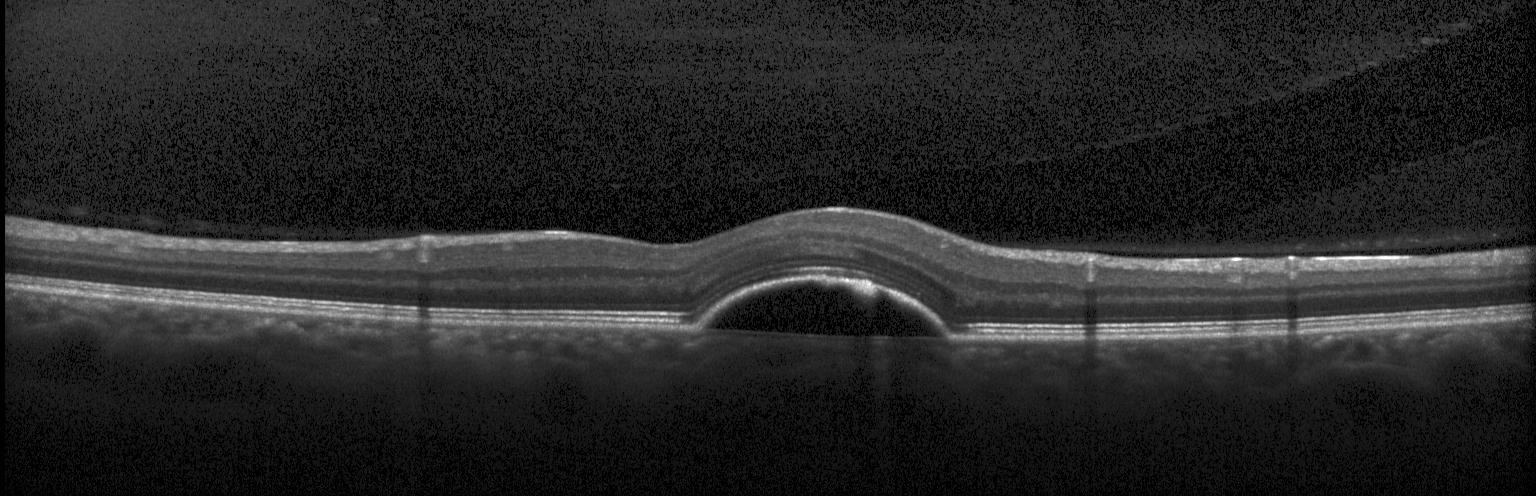
Retinal OCT B-scan, acquired on a Heidelberg Spectralis, horizontal scan through the fovea, spectral-domain OCT.
A choroidal neovascular membrane.